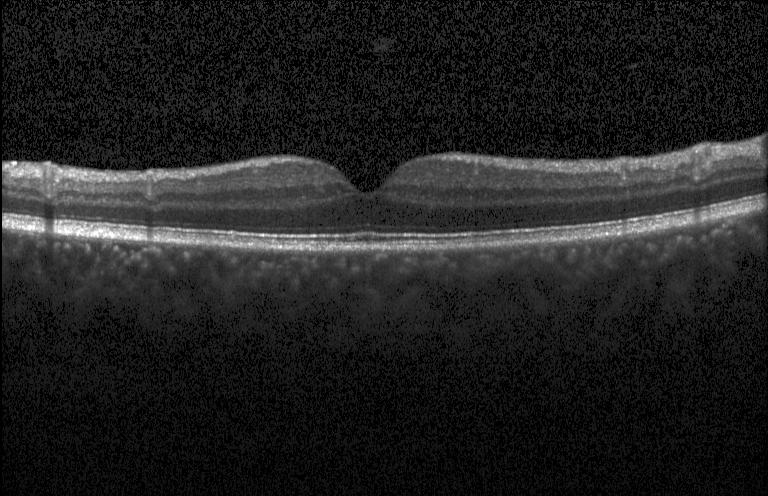

OCT line scan. Heidelberg Spectralis. Spectral-domain optical coherence tomography. Through the macula — Assessment: no evidence of CNV, DME, or drusen.